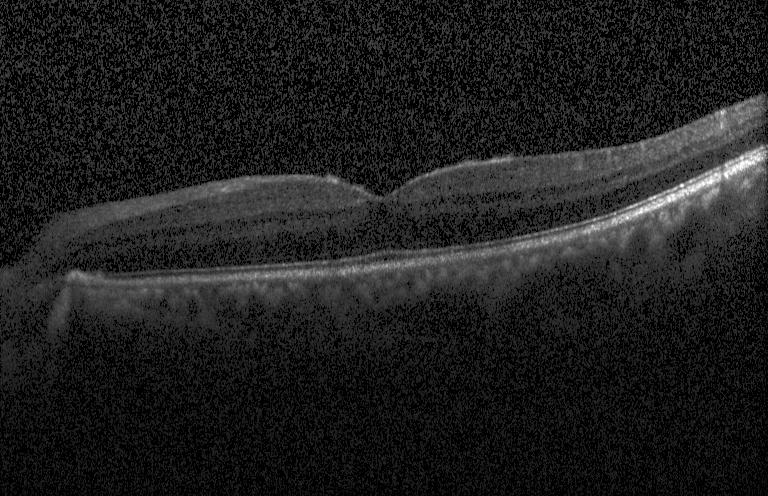

OCT B-scan. Spectral-domain optical coherence tomography. Diagnosis: no evidence of choroidal neovascularization, diabetic macular edema, or drusen.